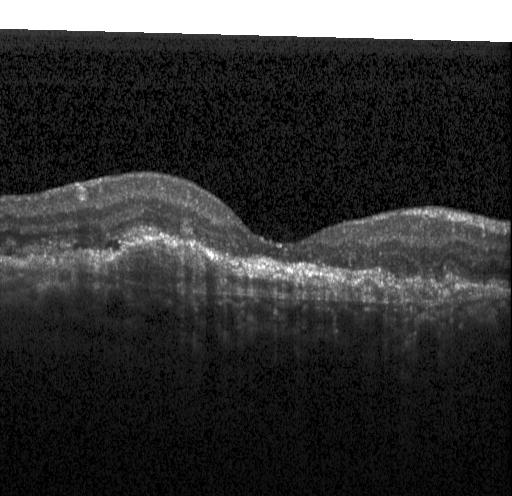
Retinal OCT cross-section — Assessment: choroidal neovascularization.